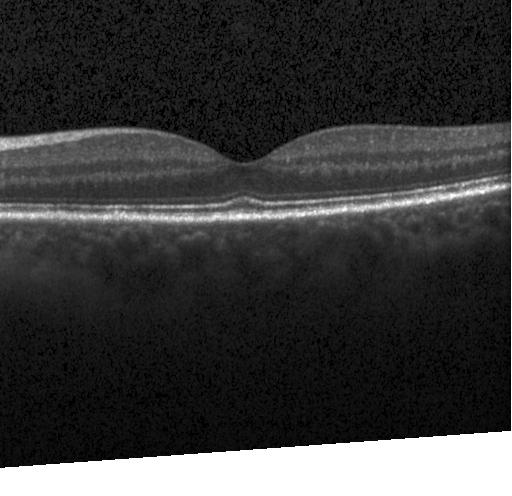 Retinal OCT B-scan.
OCT finding: neither choroidal neovascularization, diabetic macular edema, nor drusen.